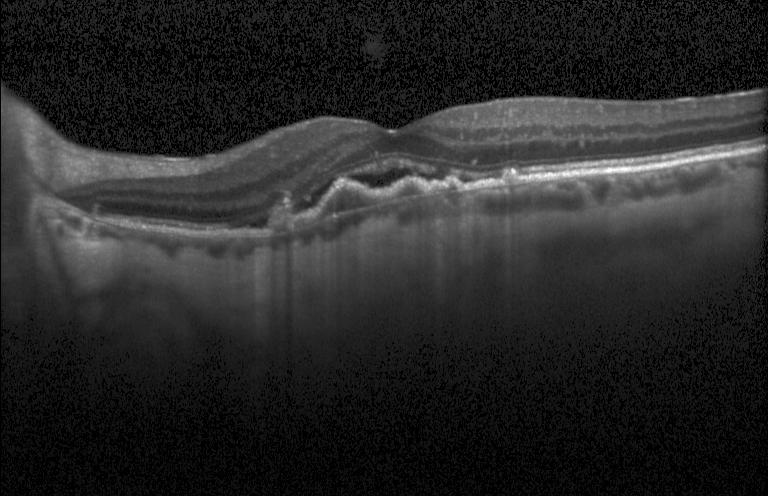 Choroidal neovascularization.